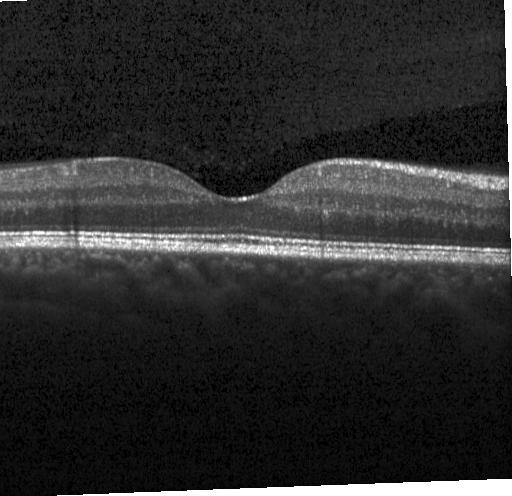

OCT B-scan showing neither choroidal neovascularization, diabetic macular edema, nor drusen.